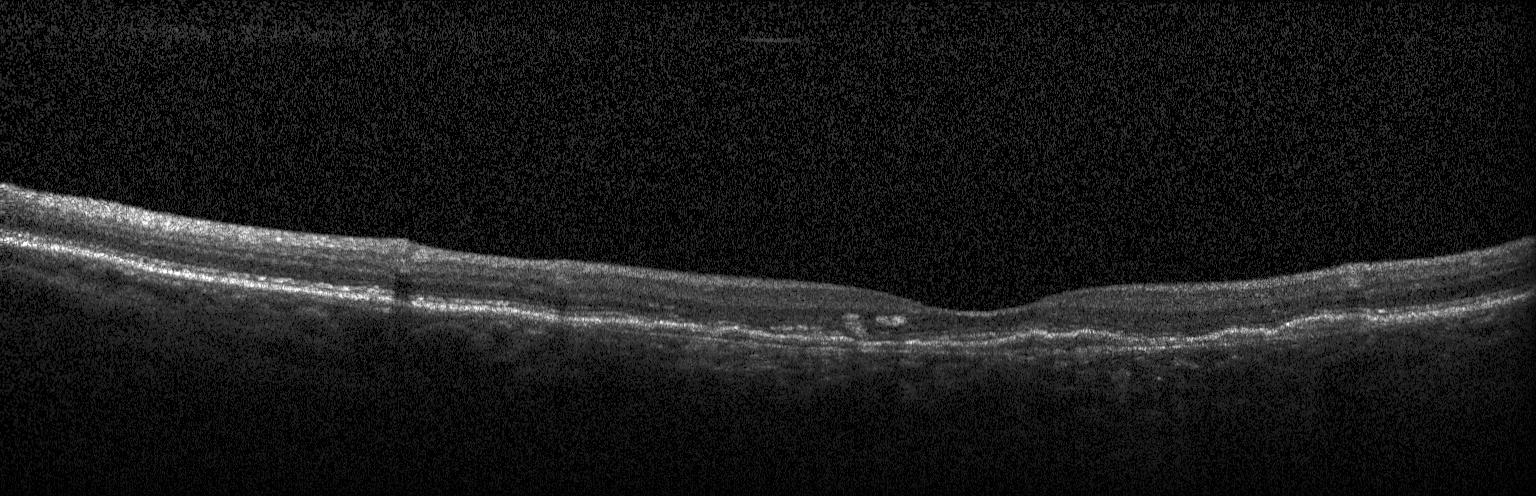 Horizontal scan through the fovea, spectral-domain OCT, OCT line scan
OCT finding: a choroidal neovascular membrane.